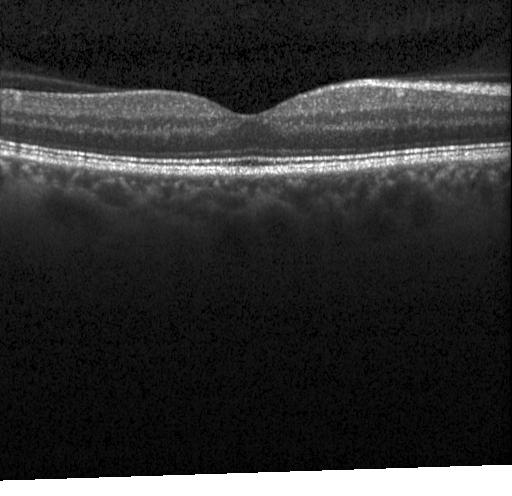
OCT B-scan.
Diagnosis: no choroidal neovascularization, no diabetic macular edema, and no drusen.